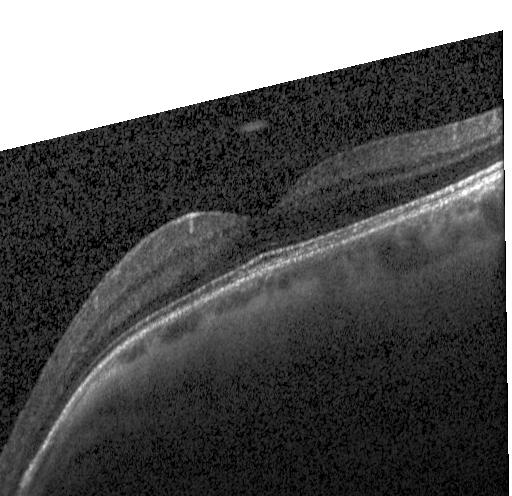
OCT line scan
Diagnosis: no CNV, DME, or drusen.